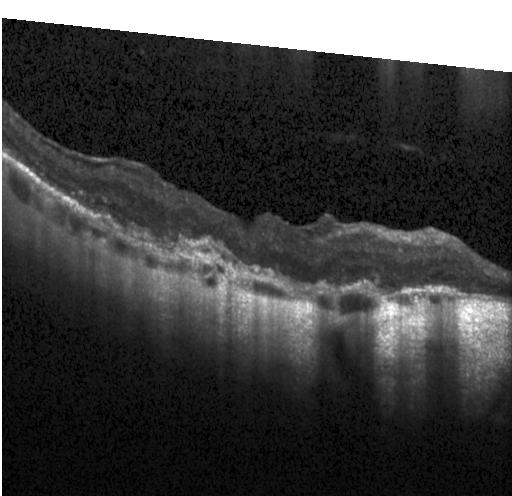

Retinal OCT cross-section showing a choroidal neovascular membrane.